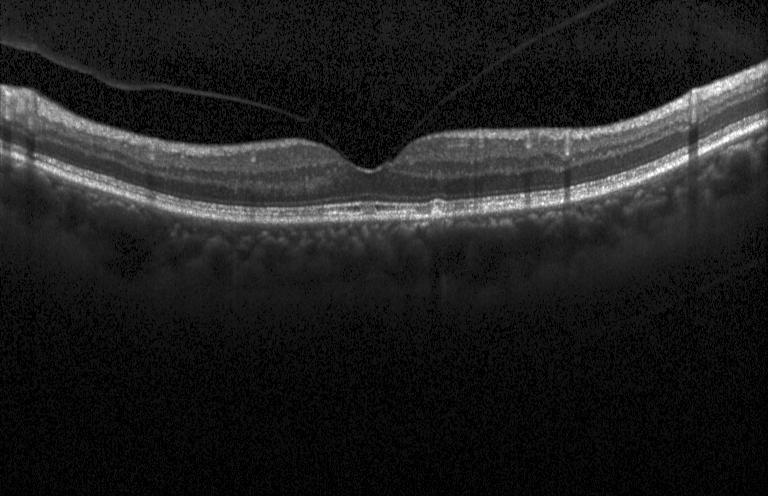

Centered on the fovea; Heidelberg Spectralis; spectral-domain optical coherence tomography; retinal OCT cross-section — Diagnosis: multiple drusen.